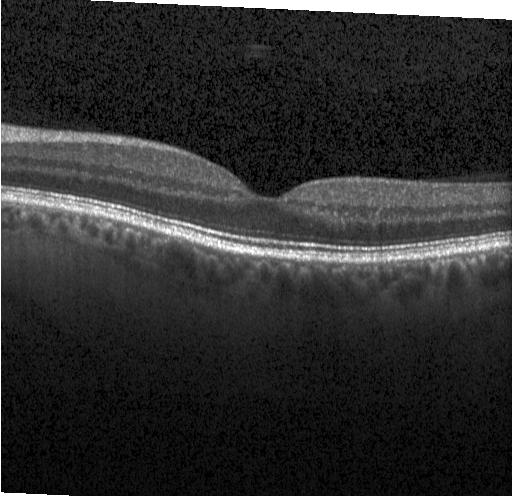
Retinal OCT B-scan · spectral-domain optical coherence tomography — Diagnosis: no choroidal neovascularization, no diabetic macular edema, and no drusen.